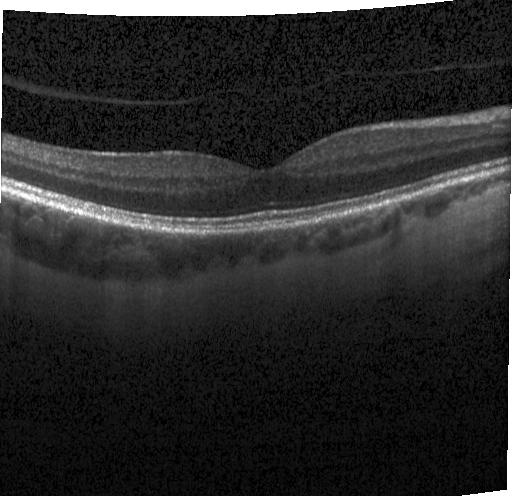 SD-OCT, retinal OCT cross-section, centered on the fovea. Impression: no evidence of CNV, DME, or drusen.